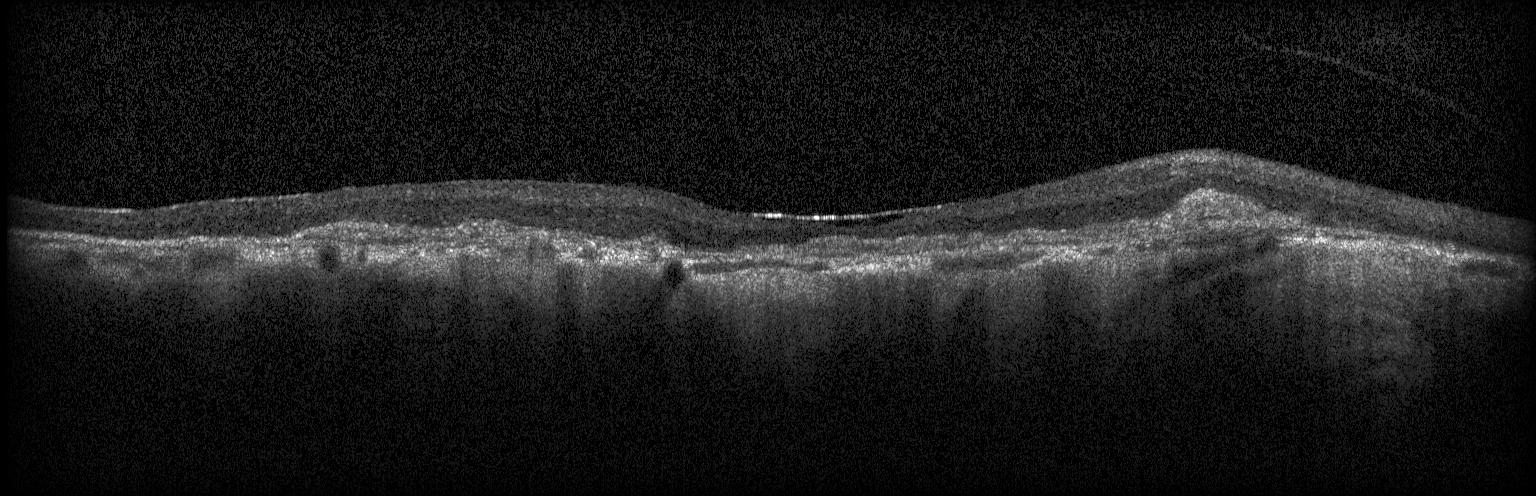
This B-scan demonstrates a choroidal neovascular membrane.